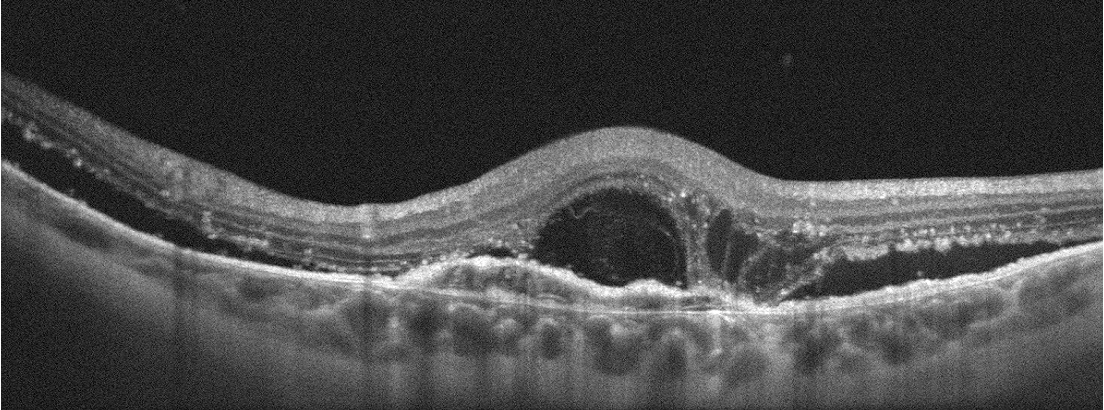

Optical coherence tomography scan.
Diagnosis: AMD.